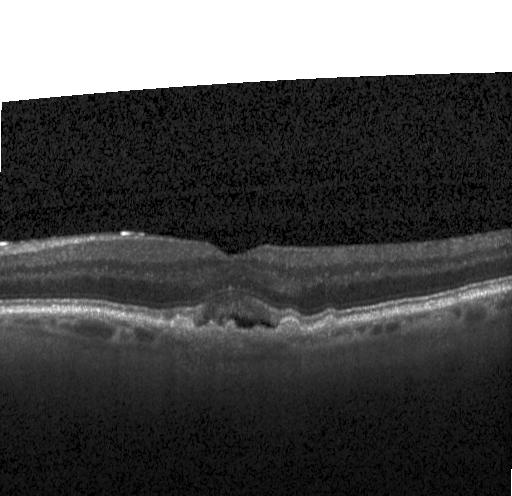 Finding: a choroidal neovascular membrane.